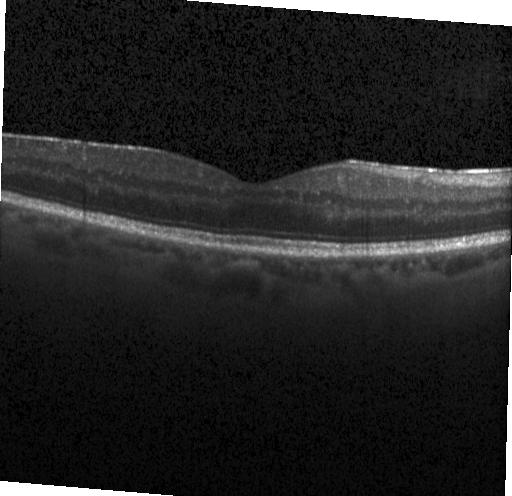 Spectral-domain optical coherence tomography, OCT B-scan.
Dx: no CNV, DME, or drusen.